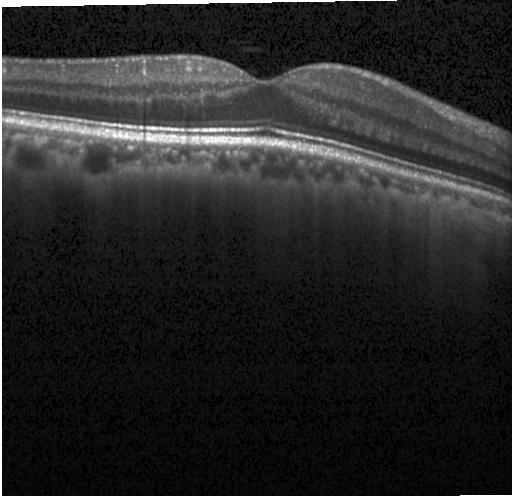

Finding: no evidence of choroidal neovascularization, diabetic macular edema, or drusen.